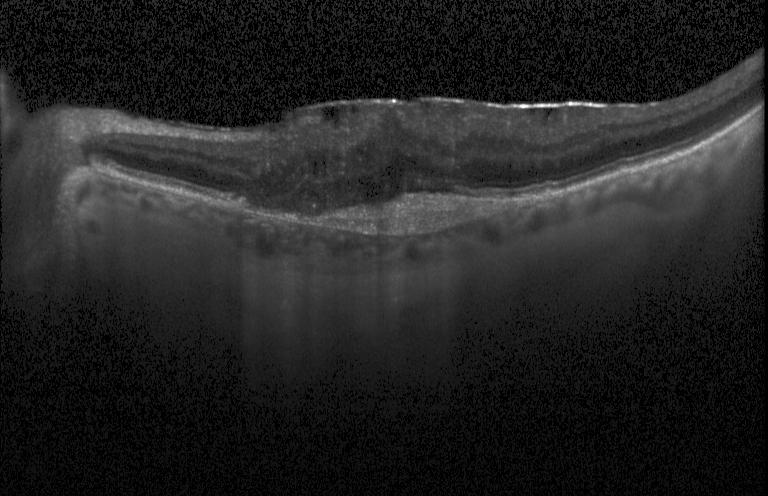
Centered on the fovea · spectral-domain OCT · optical coherence tomography B-scan.
This B-scan demonstrates a choroidal neovascular membrane.